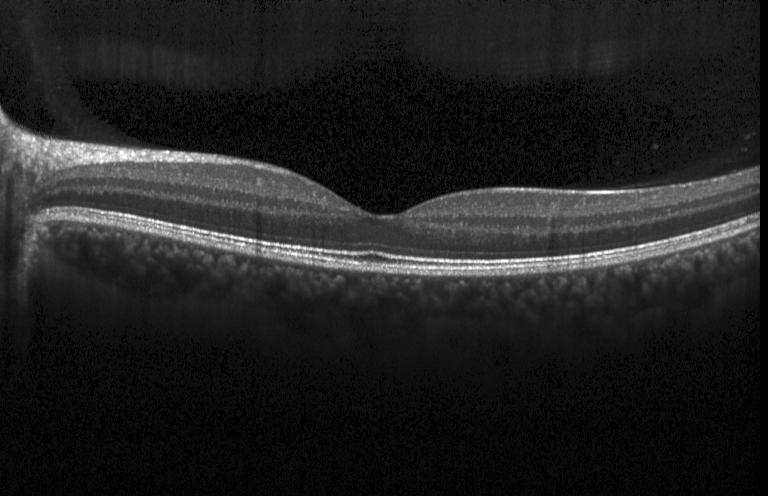 Finding: neither choroidal neovascularization, diabetic macular edema, nor drusen.